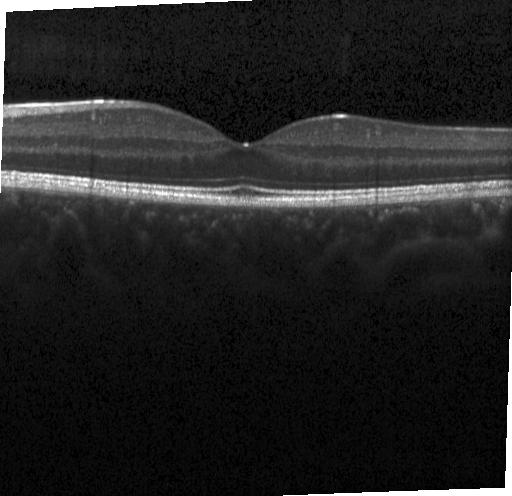 Optical coherence tomography B-scan. Finding: neither choroidal neovascularization, diabetic macular edema, nor drusen.